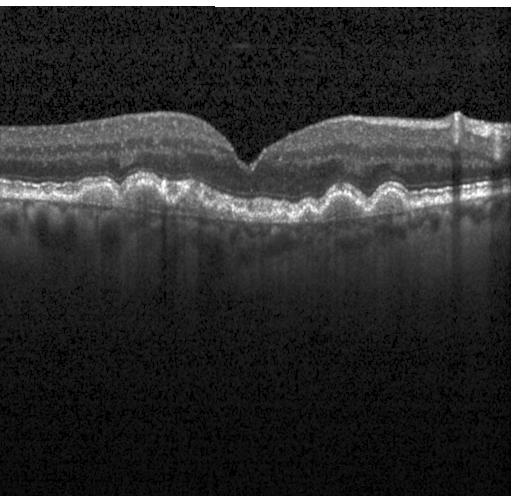 Finding: sub-RPE drusenoid deposits.